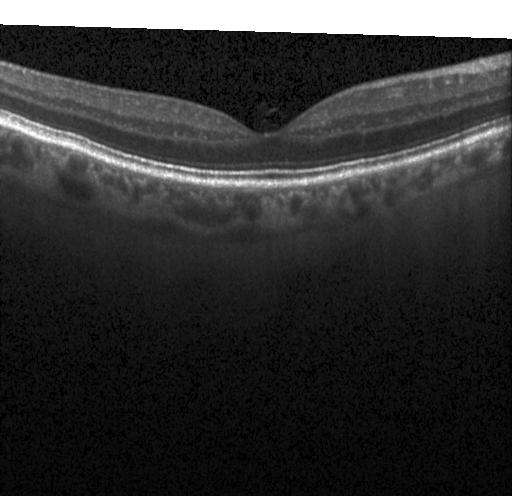
No evidence of choroidal neovascularization, diabetic macular edema, or drusen.